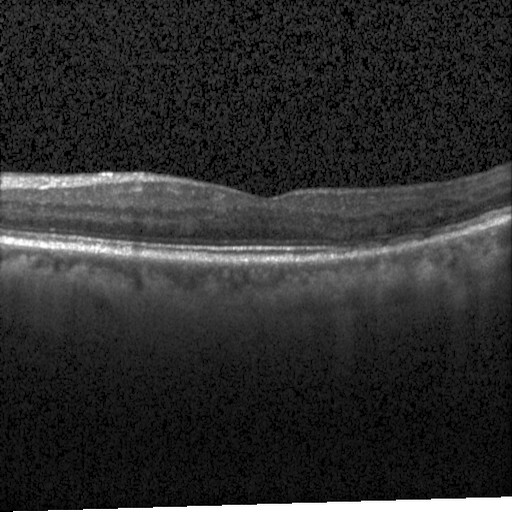 Spectral-domain OCT; optical coherence tomography B-scan; acquired on a Heidelberg Spectralis — Dx: diabetic macular edema (DME).